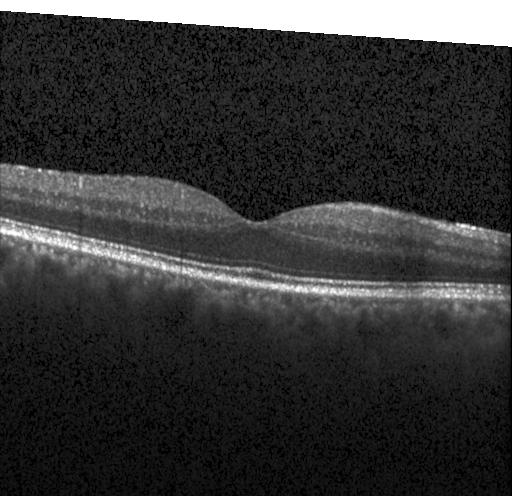

Optical coherence tomography B-scan · spectral-domain OCT · instrument: Heidelberg Spectralis.
This B-scan demonstrates no choroidal neovascularization, no diabetic macular edema, and no drusen.